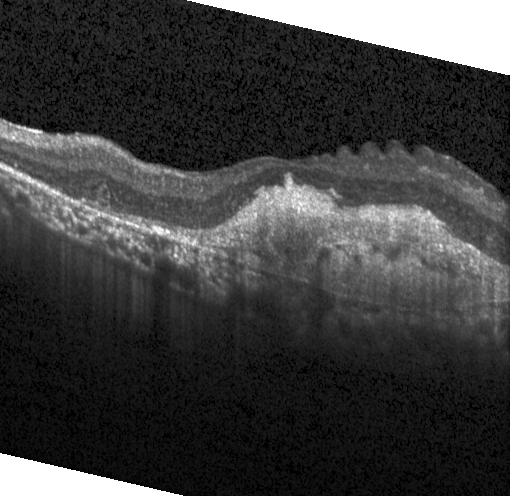 Finding: CNV.